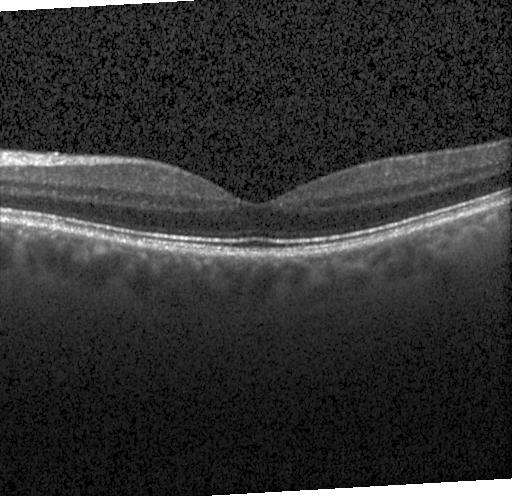
OCT line scan — Impression: no choroidal neovascularization, no diabetic macular edema, and no drusen.